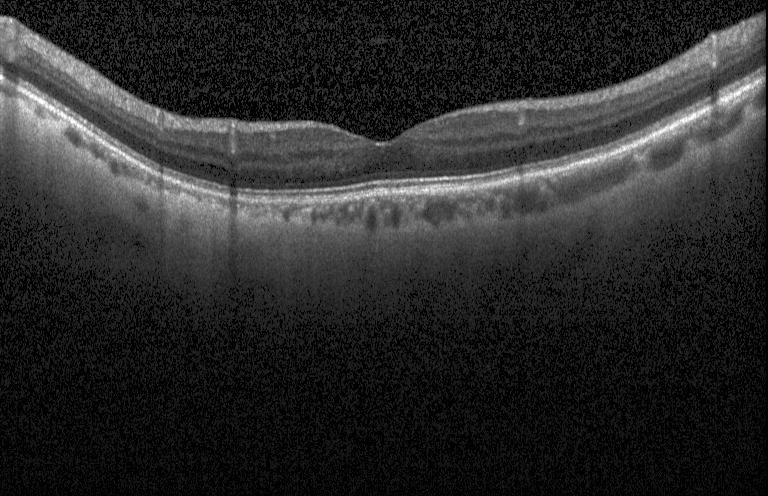

Spectral-domain optical coherence tomography · optical coherence tomography scan · Heidelberg Spectralis. Assessment: no CNV, DME, or drusen.